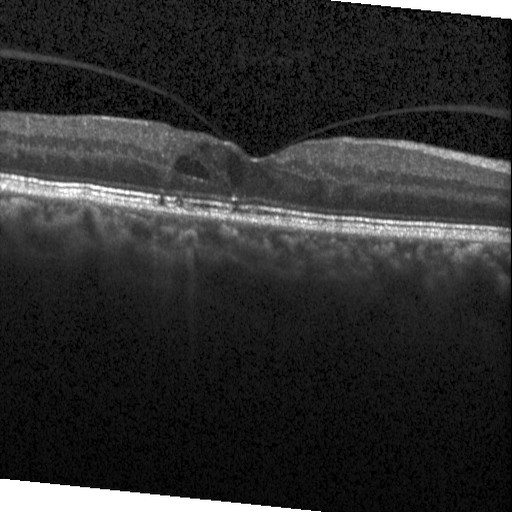

Optical coherence tomography B-scan.
DME.